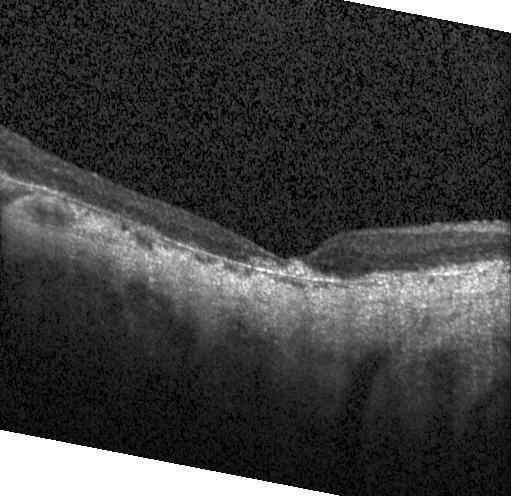
Retinal OCT B-scan, spectral-domain optical coherence tomography.
Choroidal neovascularization (CNV).